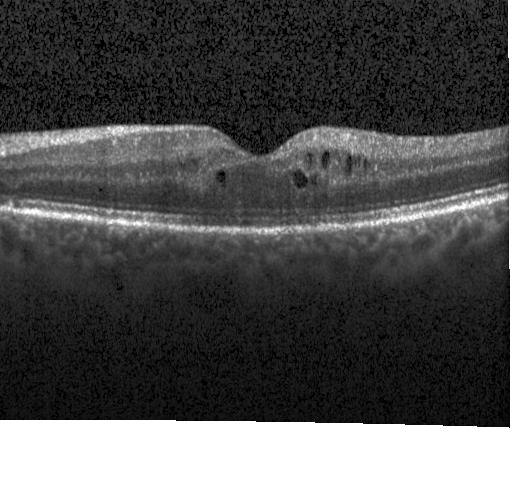

Optical coherence tomography B-scan.
Impression: diabetic macular edema (DME).